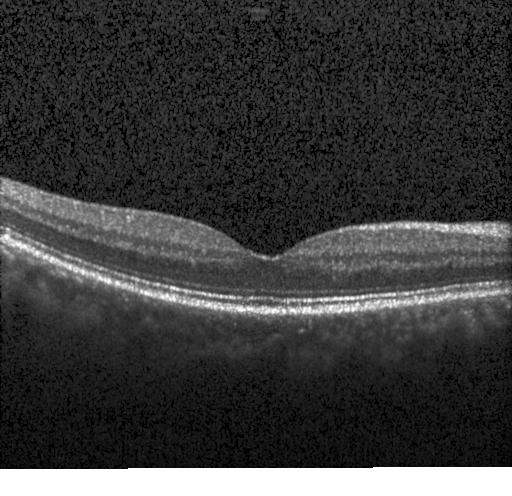 OCT B-scan. Dx: neither choroidal neovascularization, diabetic macular edema, nor drusen.